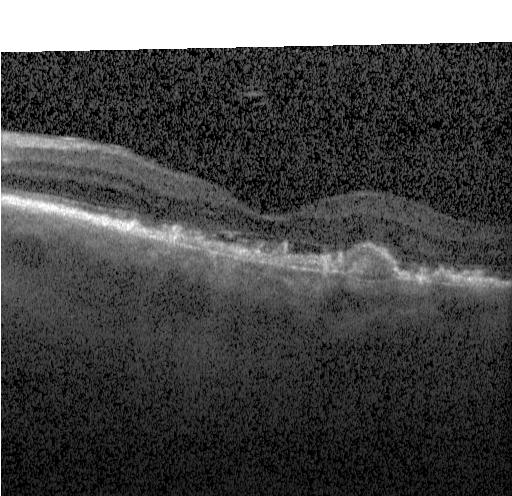 OCT B-scan.
Impression: choroidal neovascularization.